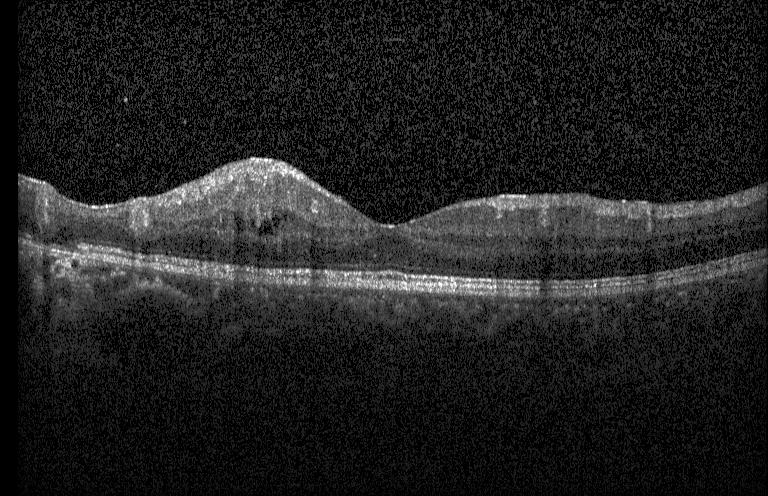

Through the macula. Heidelberg Spectralis. Retinal OCT cross-section. SD-OCT. Finding: diabetic macular edema (DME).